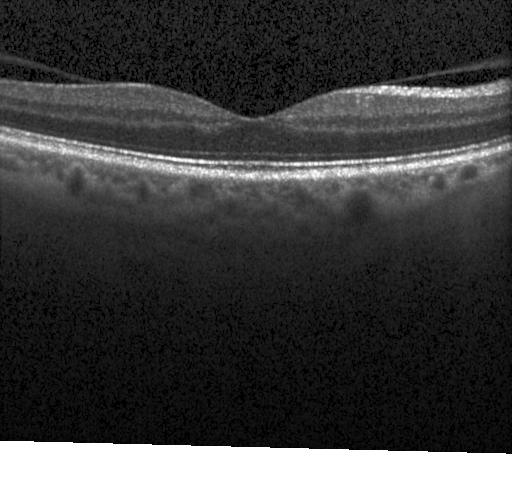

This B-scan demonstrates no choroidal neovascularization, no diabetic macular edema, and no drusen.